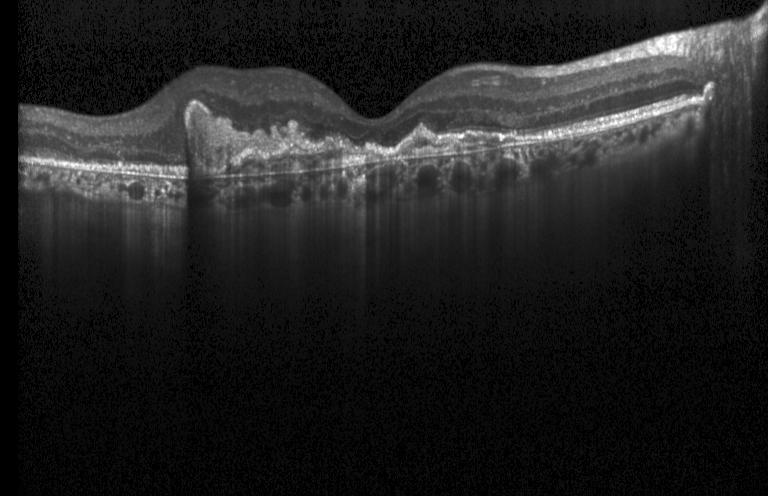
OCT B-scan
OCT finding: choroidal neovascularization (CNV).